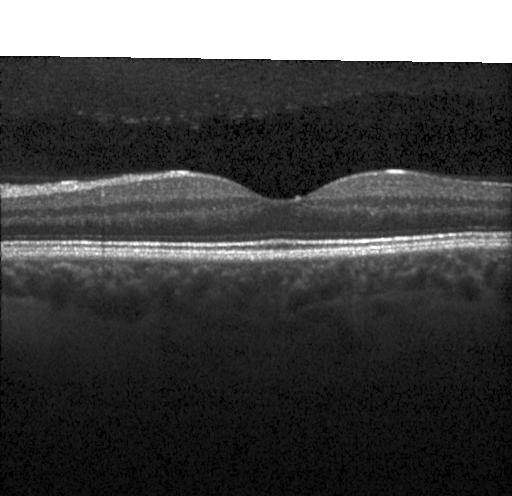
Finding: no choroidal neovascularization, no diabetic macular edema, and no drusen.